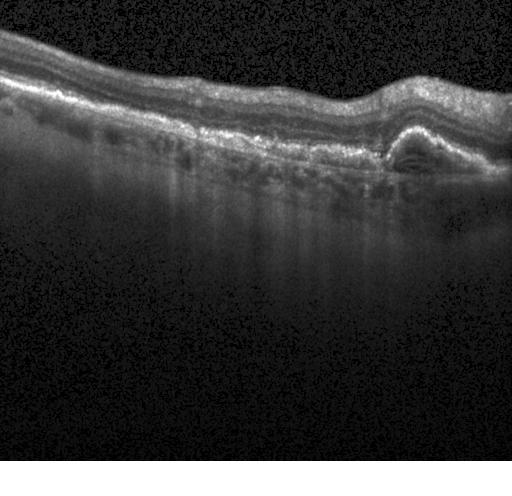
Retinal OCT cross-section
The scan shows CNV.